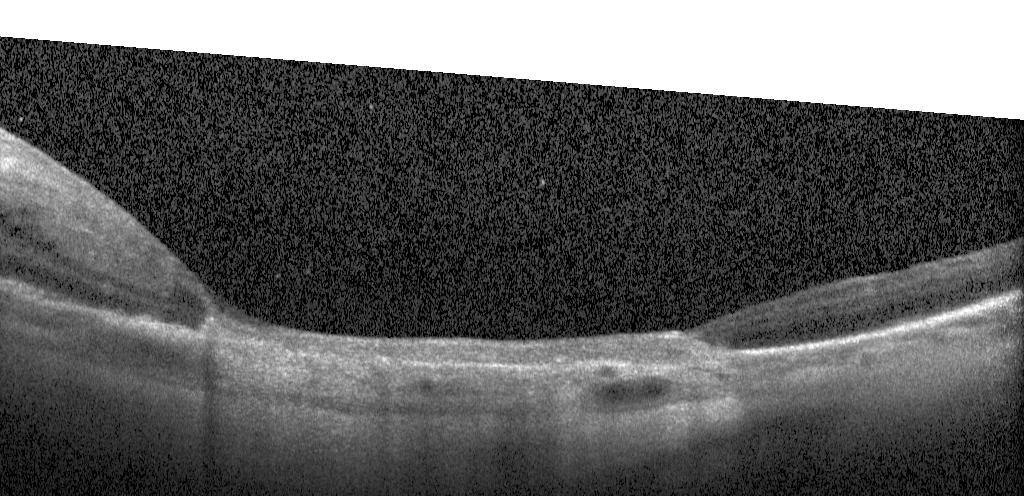 Spectral-domain optical coherence tomography; optical coherence tomography scan. Impression: choroidal neovascularization (CNV).